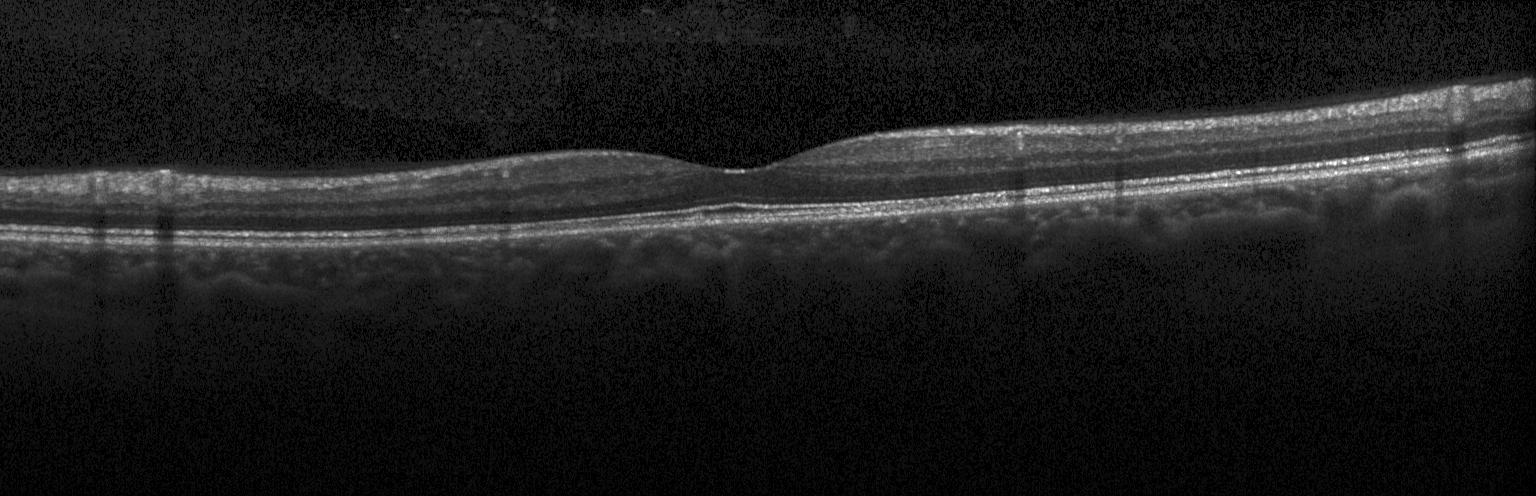
Heidelberg Spectralis · spectral-domain OCT · optical coherence tomography B-scan. Assessment: no CNV, no DME, and no drusen.